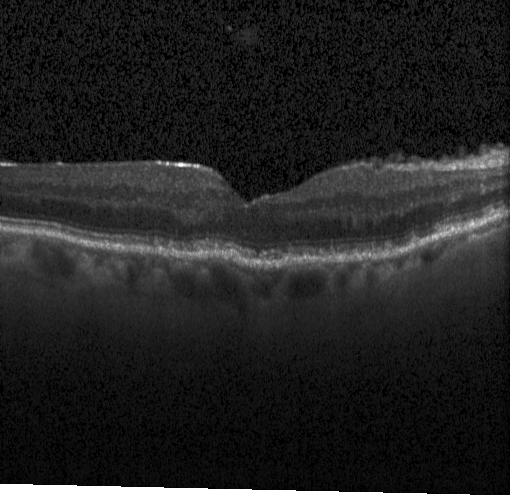

Spectral-domain OCT; retinal OCT B-scan; acquired on a Heidelberg Spectralis. Assessment: multiple drusen.